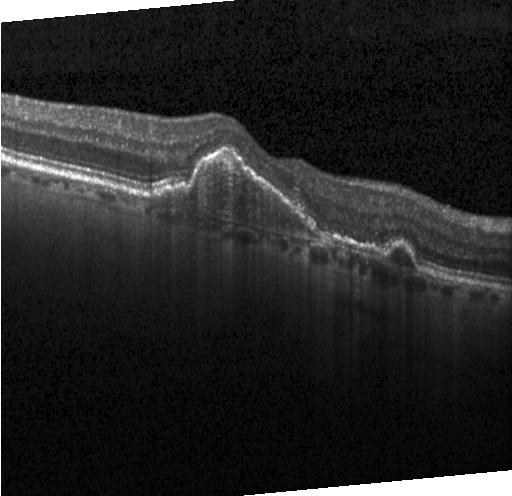 Retinal OCT cross-section, spectral-domain optical coherence tomography, fovea-centered — OCT finding: choroidal neovascularization (CNV).